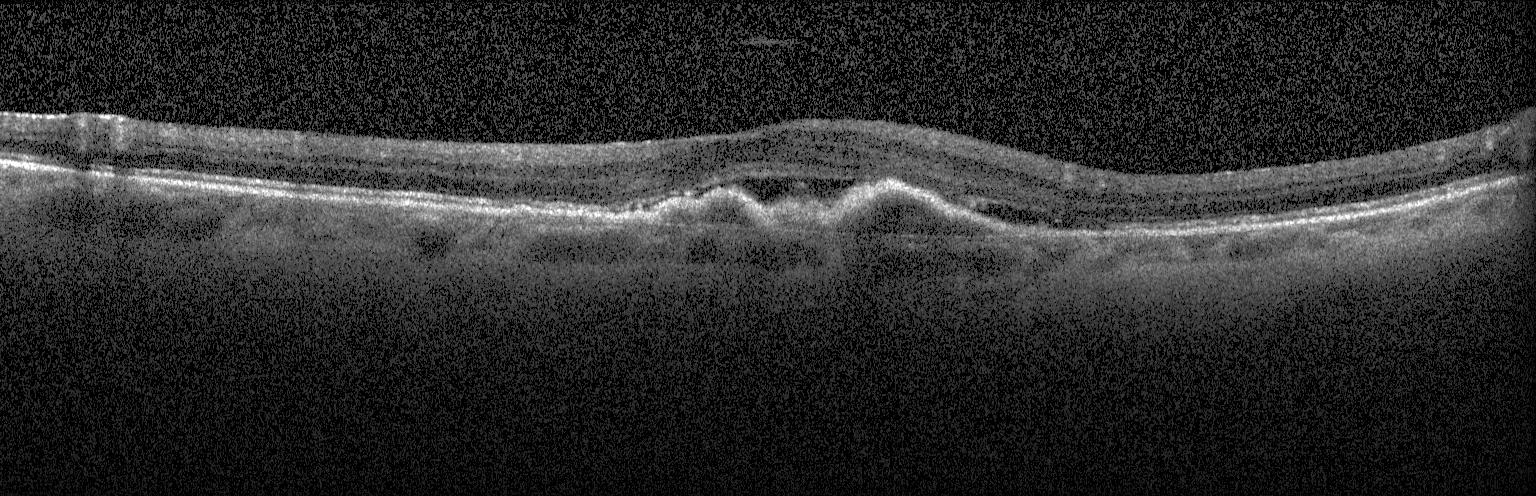

OCT scan showing choroidal neovascularization (CNV).